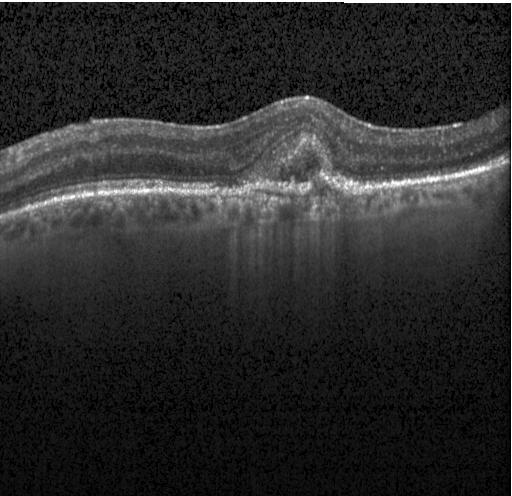

Choroidal neovascularization.